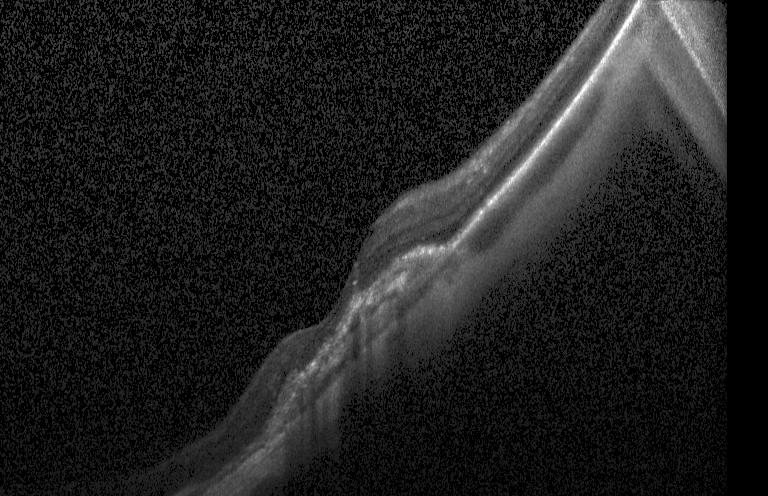 OCT finding: choroidal neovascularization (CNV).